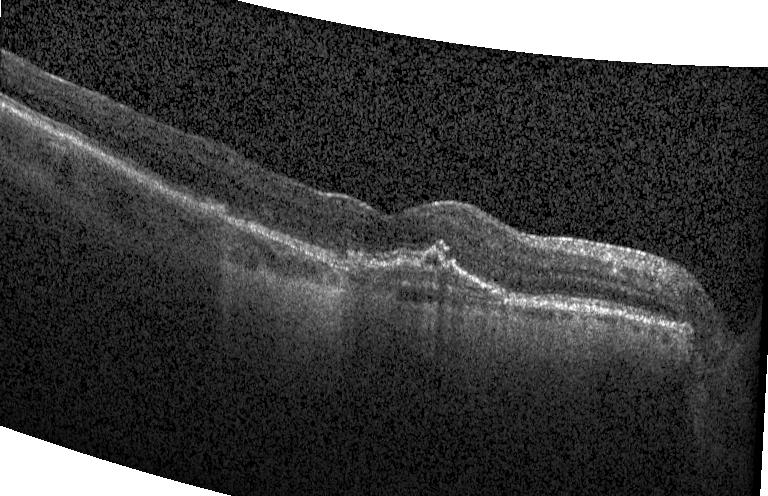

Spectral-domain OCT. Centered on the fovea. Optical coherence tomography scan
Macular OCT: CNV.